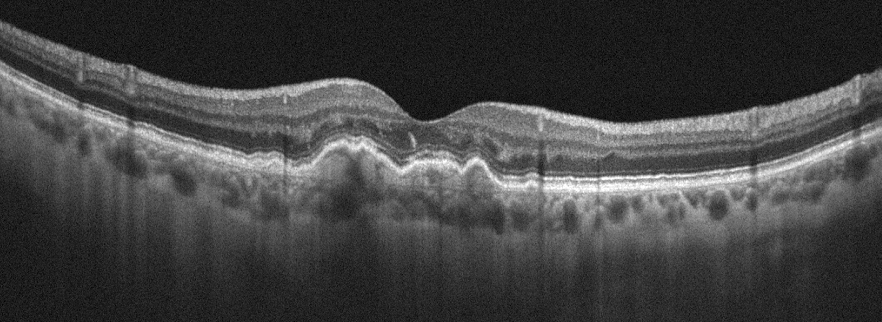

This B-scan demonstrates age-related macular degeneration (AMD).